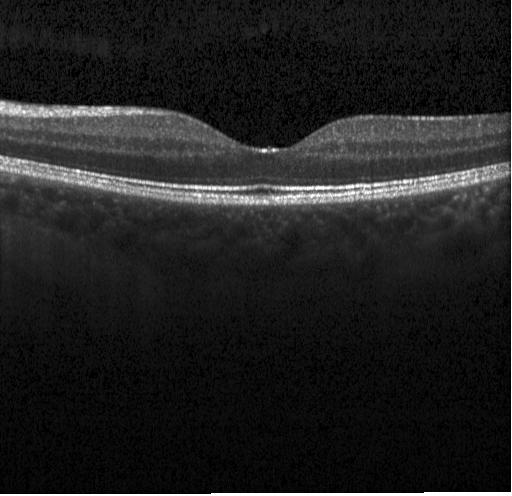
Dx: no choroidal neovascularization, no diabetic macular edema, and no drusen.